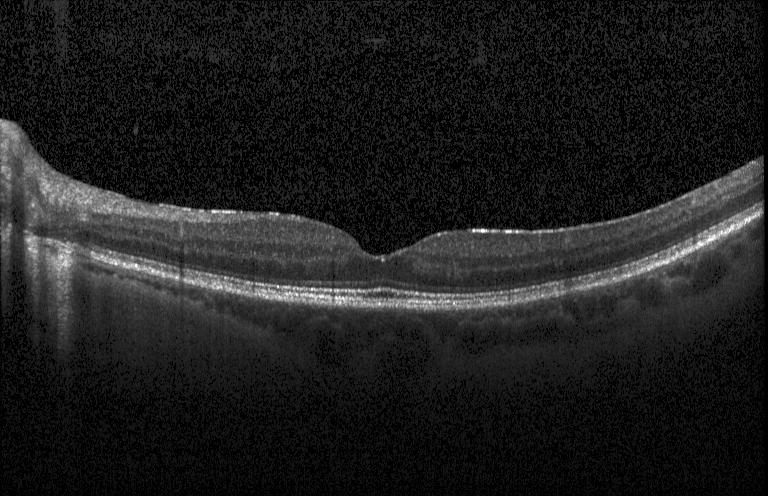

OCT line scan. Spectral-domain optical coherence tomography.
This B-scan demonstrates neither choroidal neovascularization, diabetic macular edema, nor drusen.